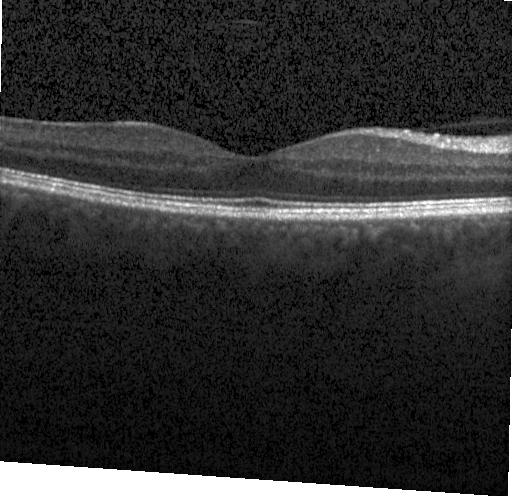

Finding: neither choroidal neovascularization, diabetic macular edema, nor drusen.